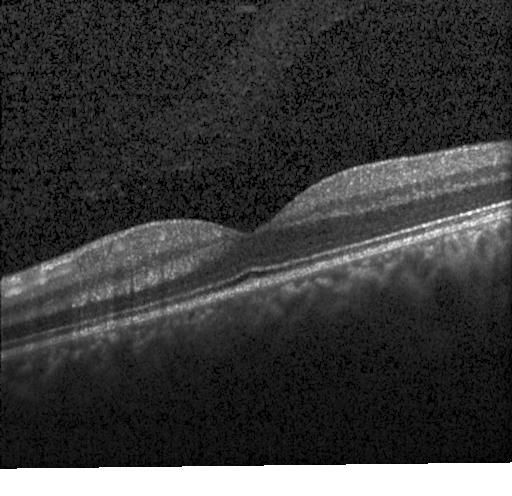
Macular scan; optical coherence tomography B-scan; Heidelberg Spectralis
Dx: neither CNV, DME, nor drusen.